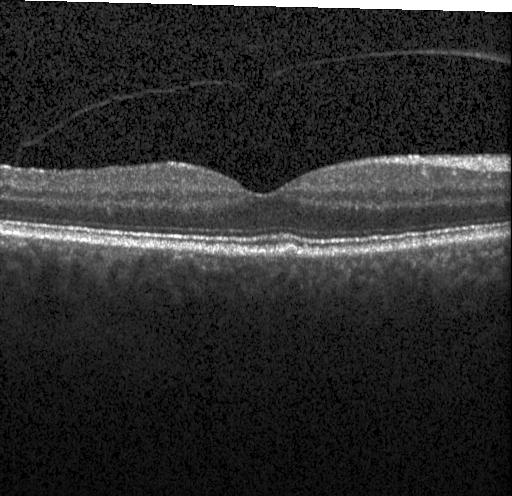 Macular scan · spectral-domain OCT · optical coherence tomography scan.
Impression: multiple drusen.